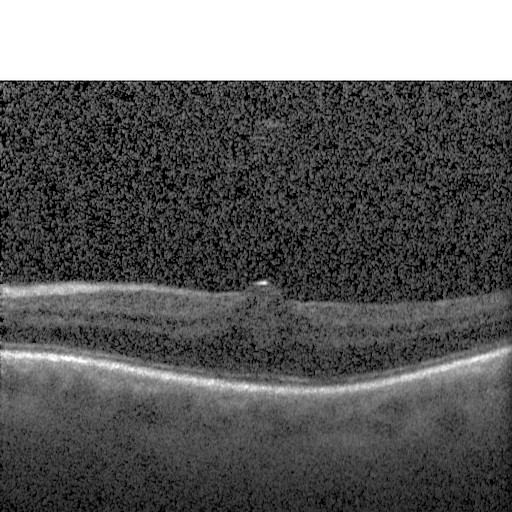

Impression: DME.